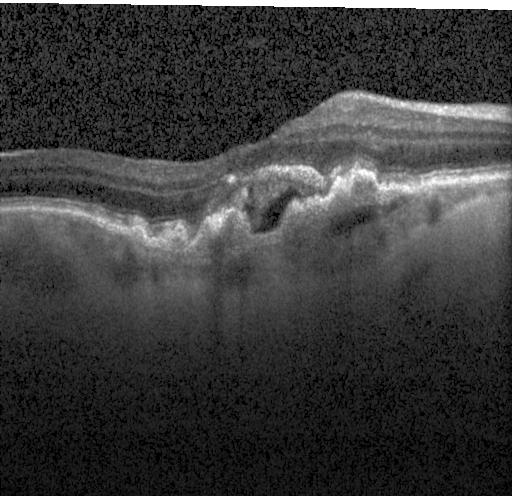 Centered on the fovea. Optical coherence tomography scan. Assessment: CNV.